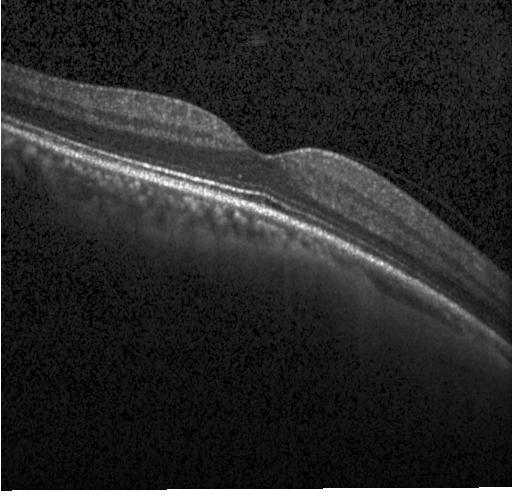
Centered on the fovea, retinal OCT B-scan, SD-OCT, instrument: Heidelberg Spectralis — Finding: neither choroidal neovascularization, diabetic macular edema, nor drusen.